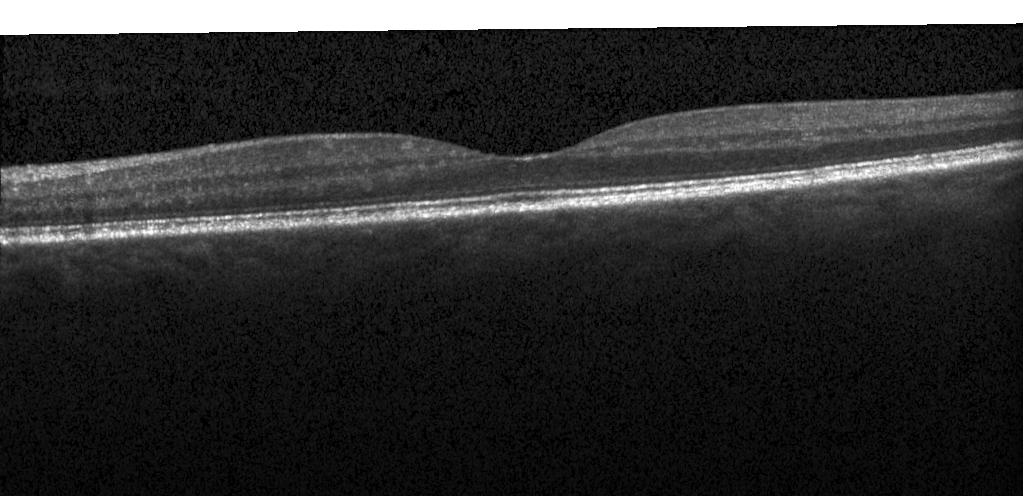

Acquired on a Heidelberg Spectralis. Retinal OCT B-scan. Impression: no choroidal neovascularization, no diabetic macular edema, and no drusen.